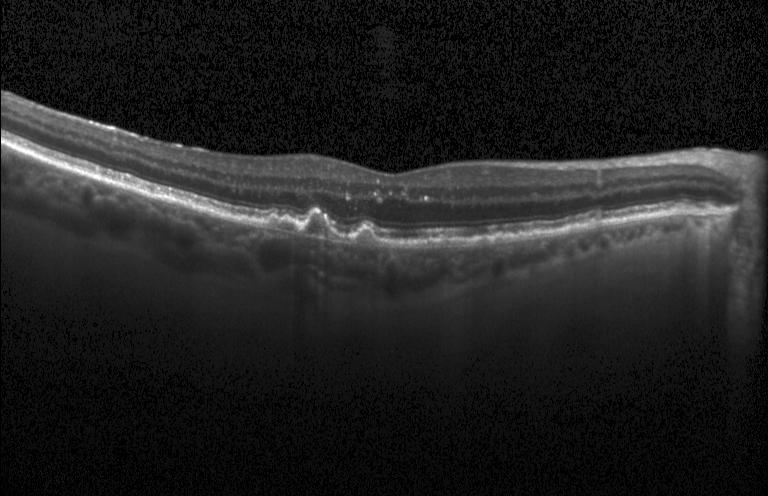
Retinal OCT cross-section showing sub-RPE drusenoid deposits.